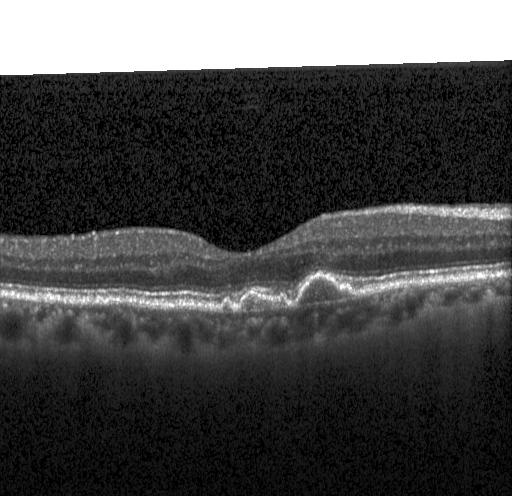 Heidelberg Spectralis OCT system. OCT B-scan
Impression: multiple drusen.